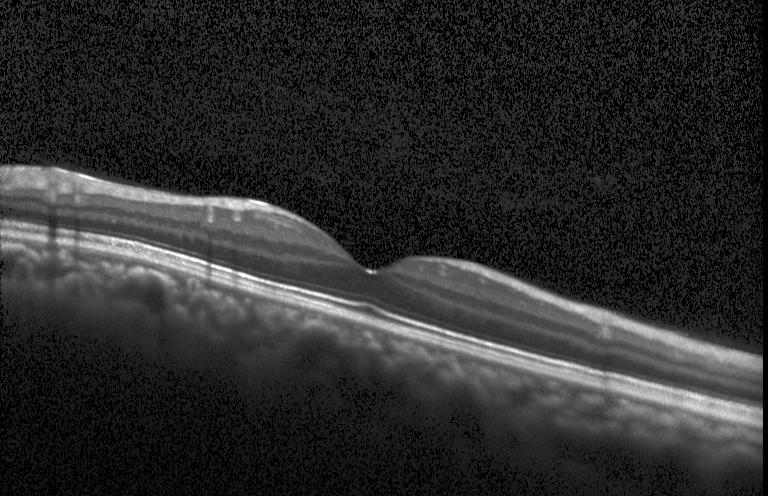
No evidence of choroidal neovascularization, diabetic macular edema, or drusen.